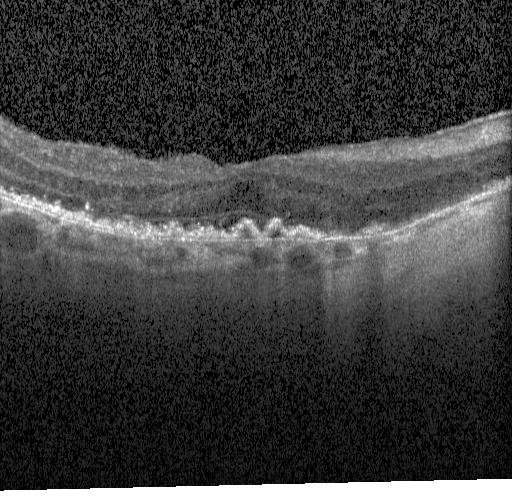

OCT line scan.
Impression: a choroidal neovascular membrane.